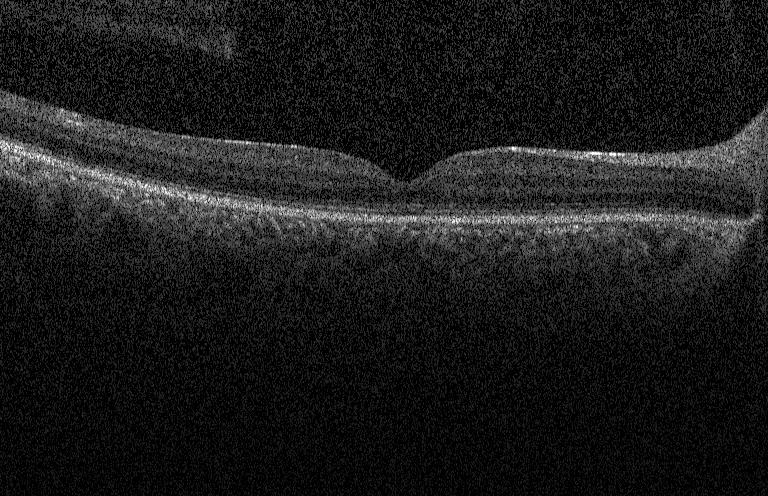 Retinal OCT cross-section; Heidelberg Spectralis — The scan shows no evidence of choroidal neovascularization, diabetic macular edema, or drusen.